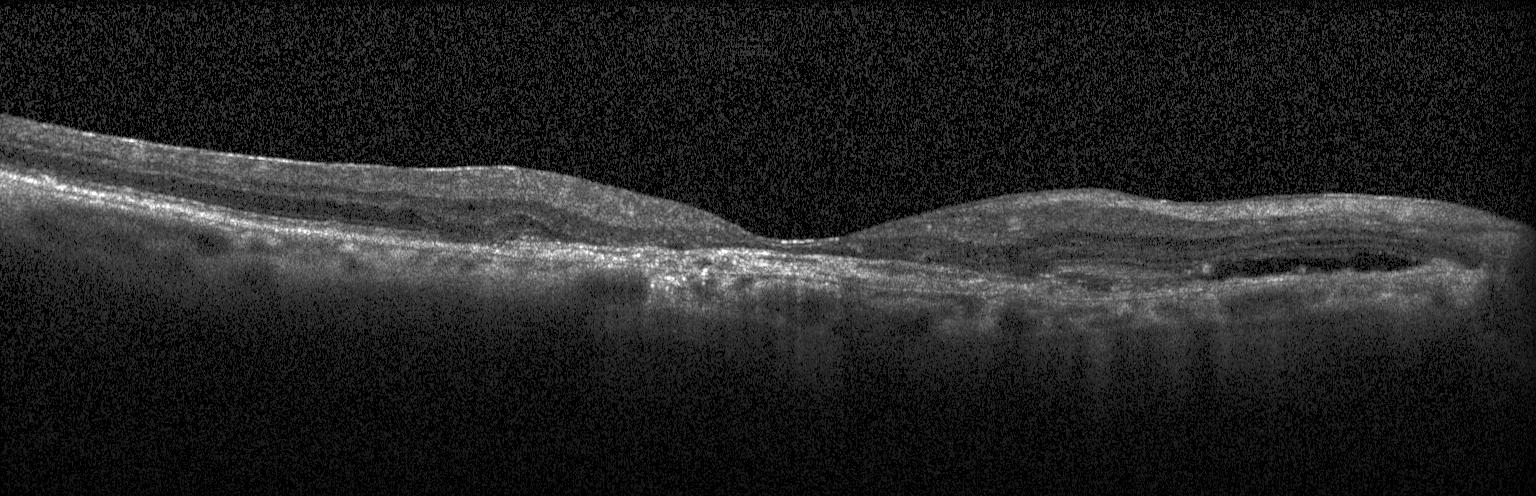
Instrument: Heidelberg Spectralis. Retinal OCT B-scan — Assessment: choroidal neovascularization.